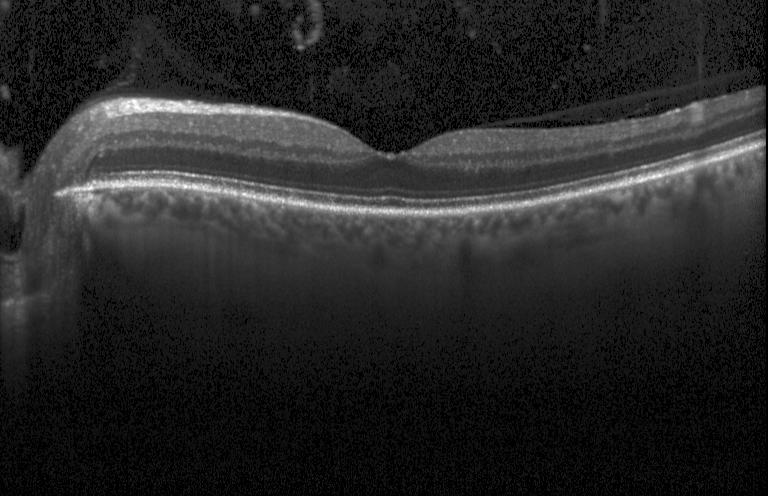
Acquired on a Heidelberg Spectralis, OCT line scan — OCT finding: no evidence of CNV, DME, or drusen.